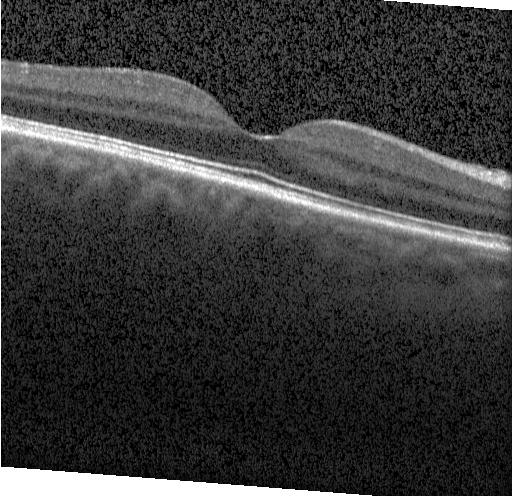
Spectral-domain OCT · acquired on a Heidelberg Spectralis · through the macula · retinal OCT cross-section — Impression: no evidence of CNV, DME, or drusen.